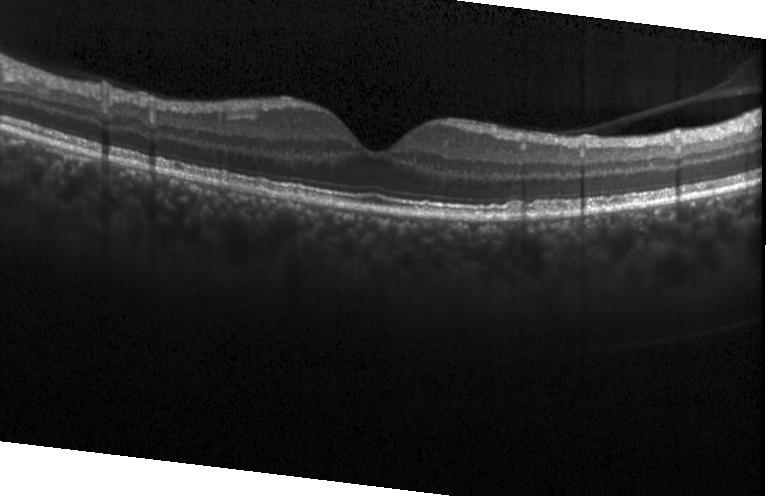
Optical coherence tomography B-scan.
Finding: multiple drusen.